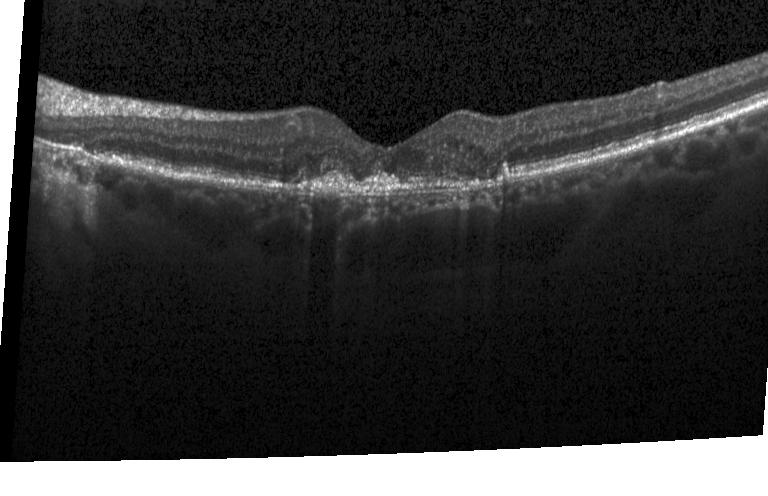

Heidelberg Spectralis OCT system, macular scan, OCT B-scan, spectral-domain optical coherence tomography. Diagnosis: a choroidal neovascular membrane.